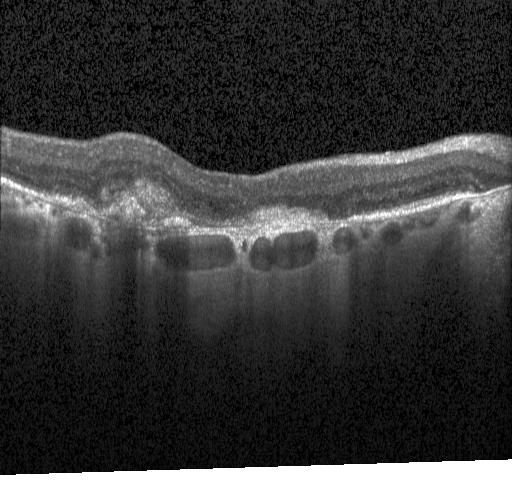
Spectral-domain optical coherence tomography · instrument: Heidelberg Spectralis · OCT B-scan. Assessment: a choroidal neovascular membrane.